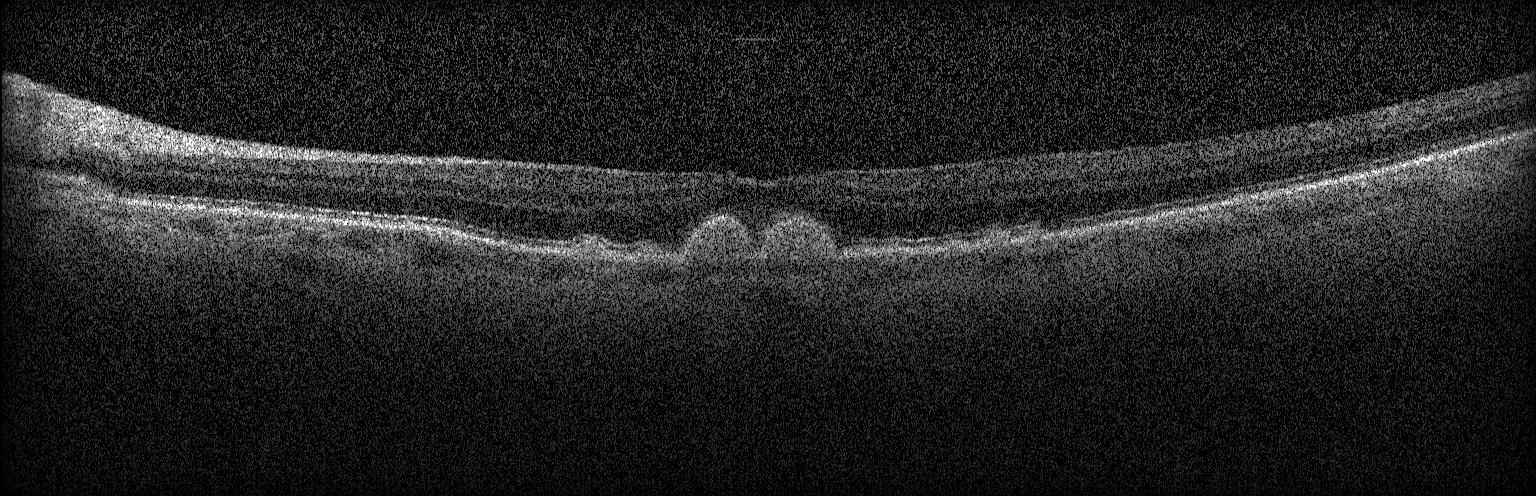

Finding: drusen.